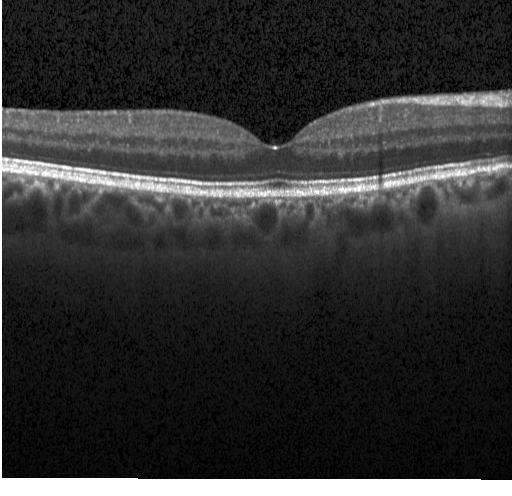 Optical coherence tomography scan. Impression: no choroidal neovascularization, diabetic macular edema, or drusen.